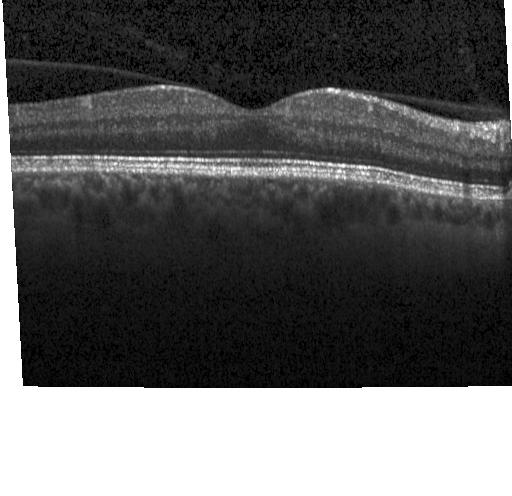
Retinal OCT cross-section showing no evidence of CNV, DME, or drusen.